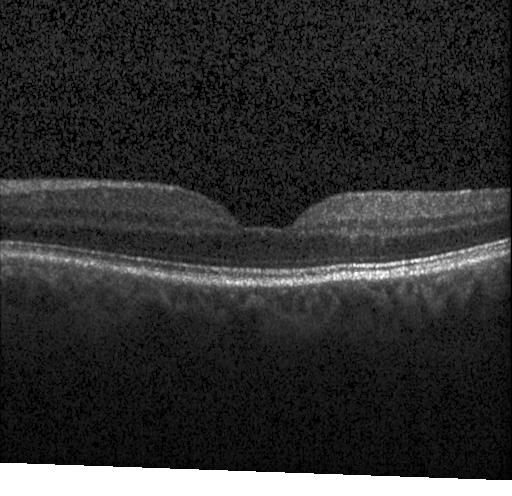
Optical coherence tomography B-scan. Heidelberg Spectralis.
Macular OCT: no choroidal neovascularization, no diabetic macular edema, and no drusen.